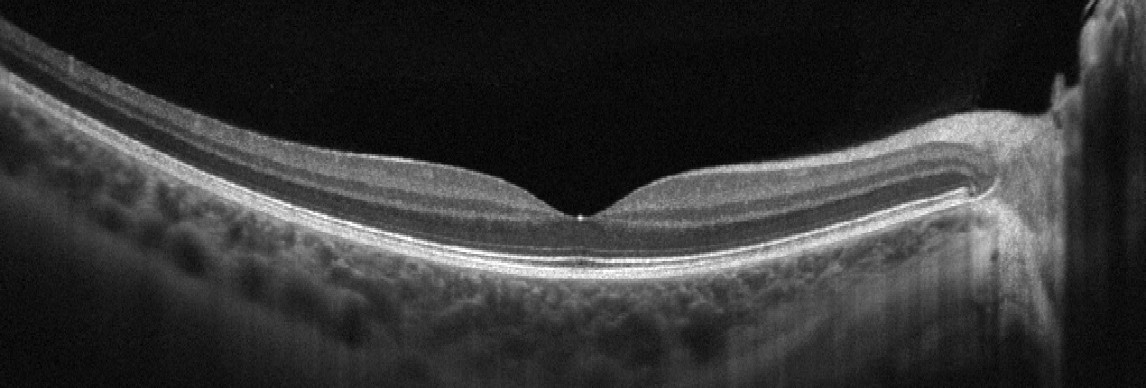

No evidence of AMD, DME, ERM, RAO, RVO, or VID.